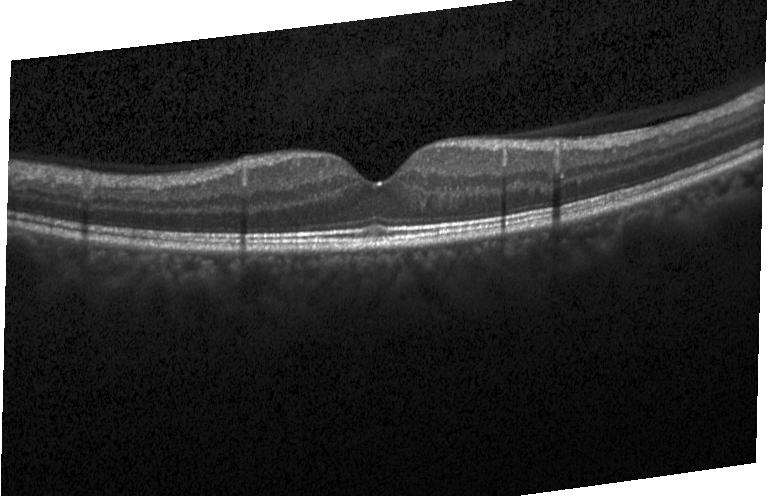

Optical coherence tomography scan — Macular OCT: no evidence of choroidal neovascularization, diabetic macular edema, or drusen.